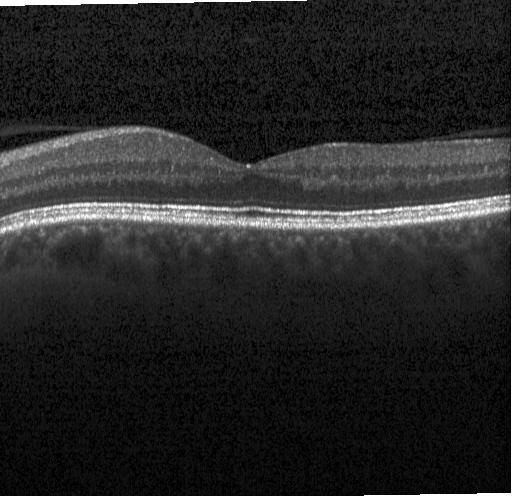 OCT line scan. Heidelberg Spectralis OCT system. Fovea-centered — Dx: no evidence of choroidal neovascularization, diabetic macular edema, or drusen.